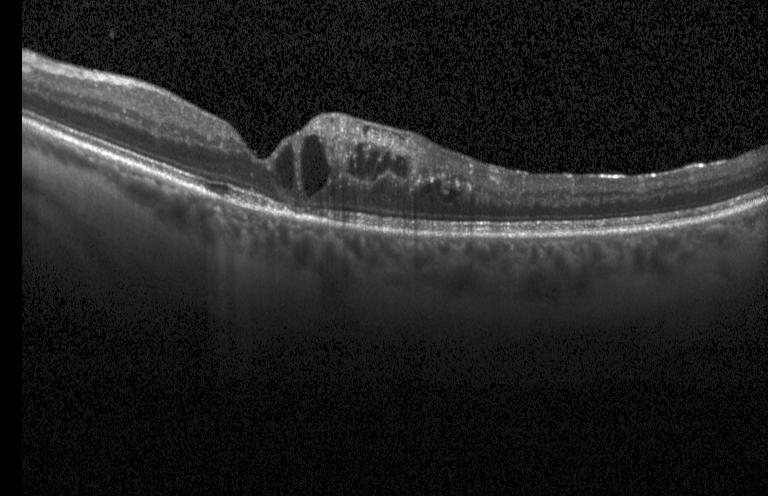 OCT finding: DME.